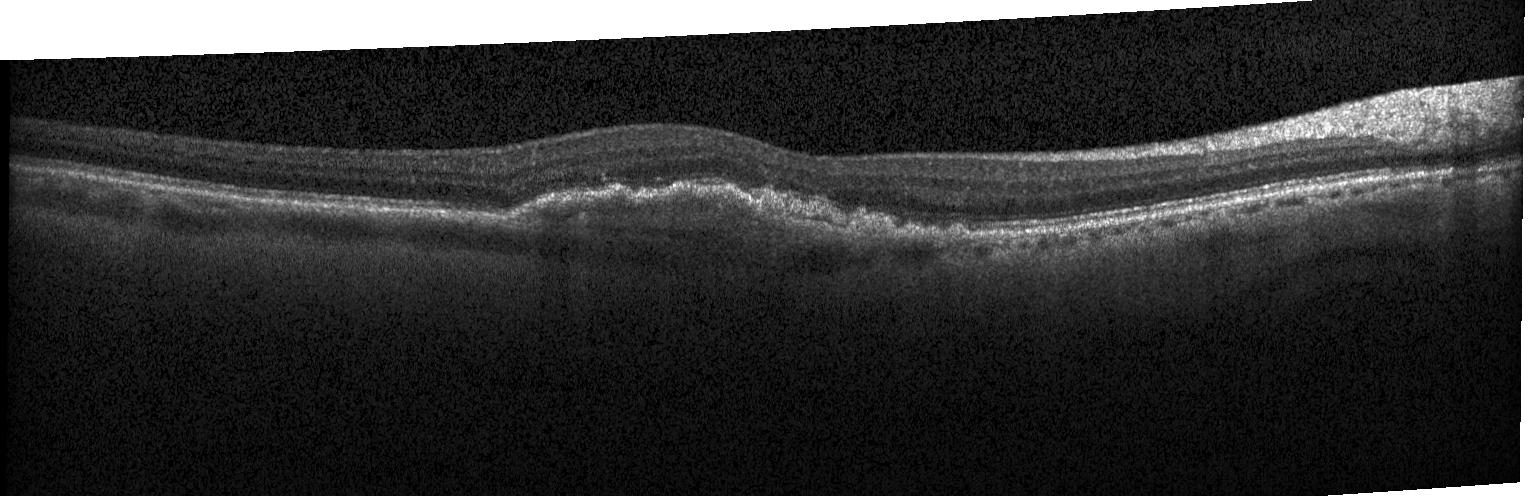 Horizontal scan through the fovea · OCT line scan · SD-OCT.
Diagnosis: choroidal neovascularization (CNV).